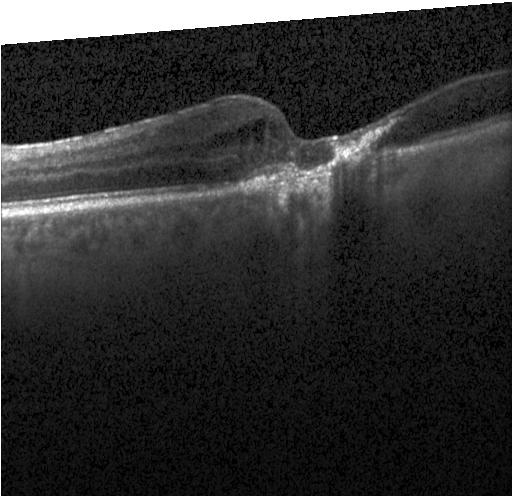 Diagnosis: choroidal neovascularization (CNV).